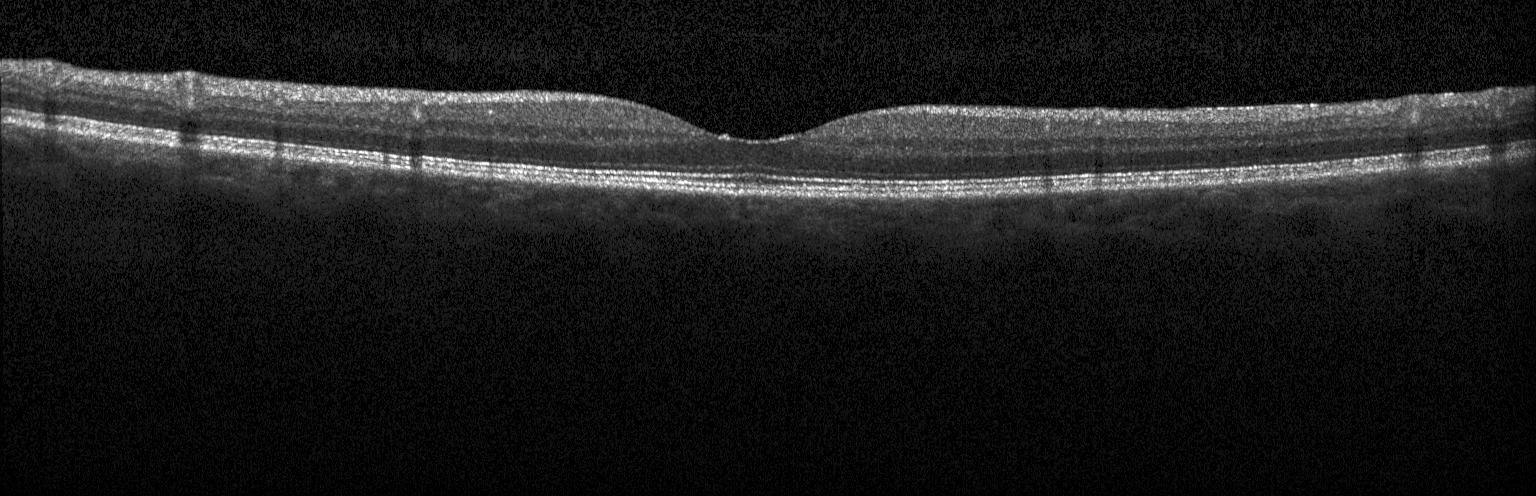 Retinal OCT cross-section showing no choroidal neovascularization, diabetic macular edema, or drusen.